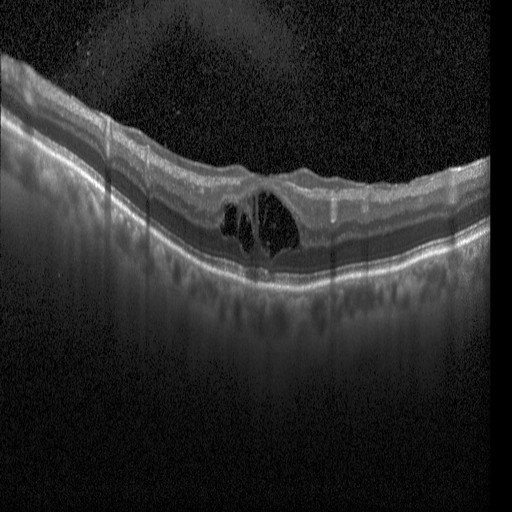

This B-scan demonstrates diabetic macular edema.